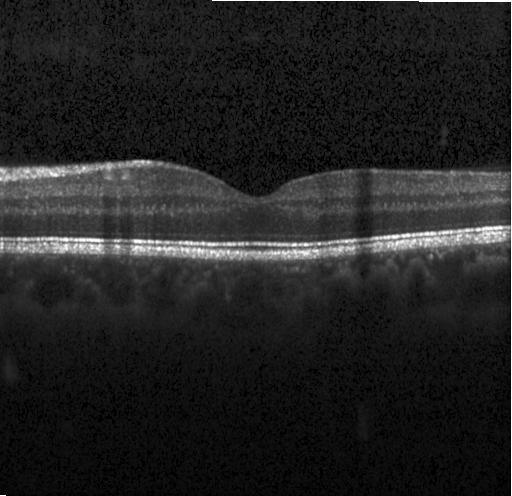
OCT B-scan.
Assessment: neither CNV, DME, nor drusen.